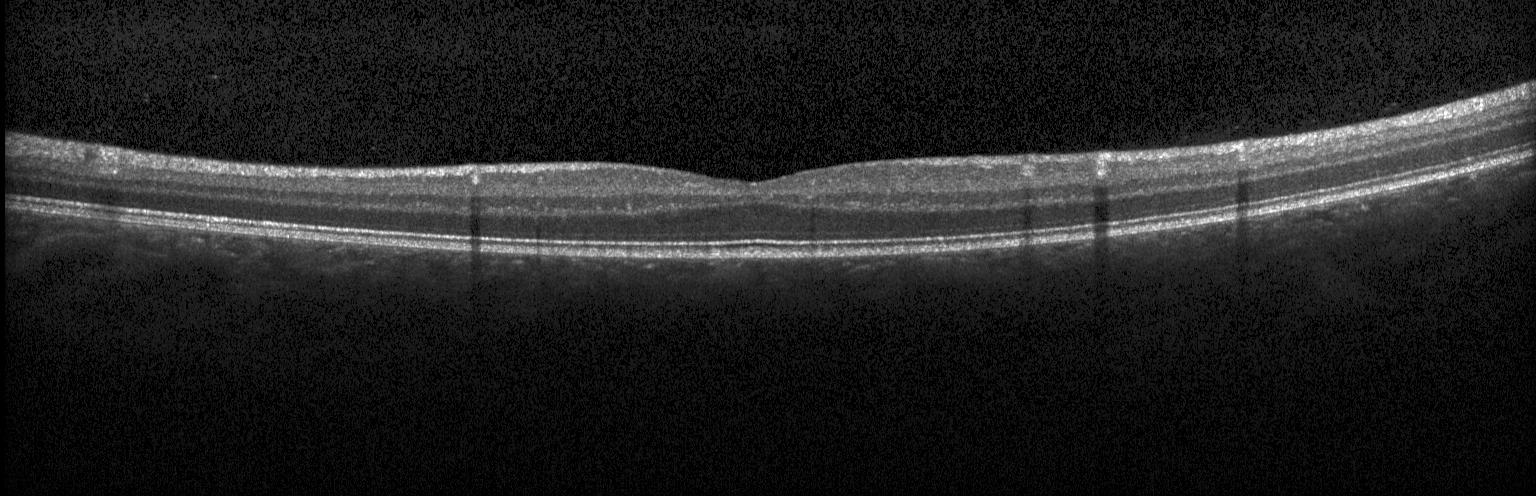

Heidelberg Spectralis OCT system · OCT line scan.
The scan shows neither choroidal neovascularization, diabetic macular edema, nor drusen.